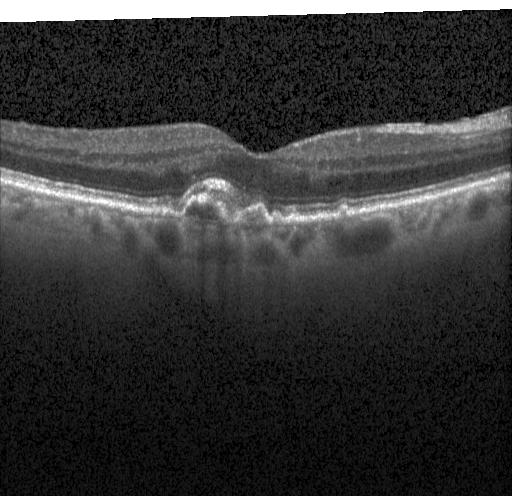

Fovea-centered, acquired on a Heidelberg Spectralis, retinal OCT B-scan.
The scan shows a choroidal neovascular membrane.